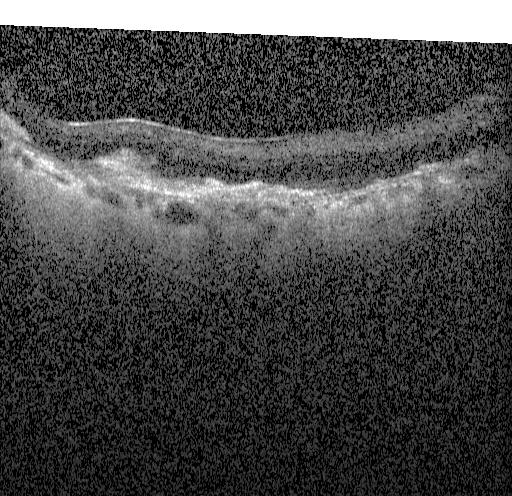 OCT finding: a choroidal neovascular membrane.